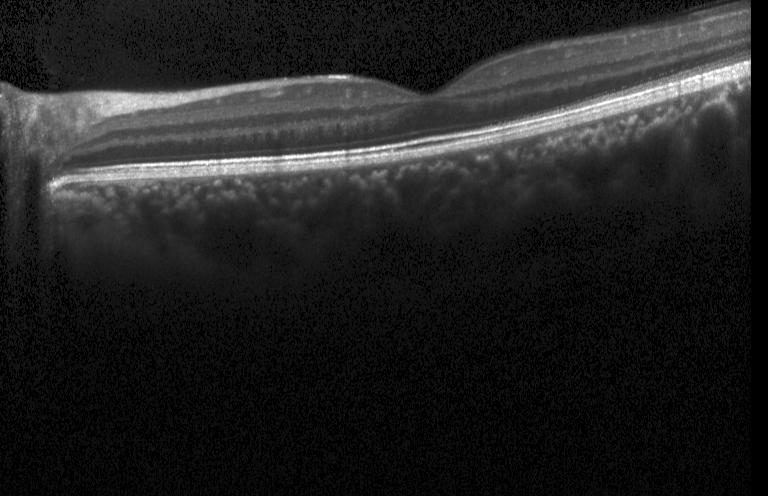 OCT B-scan · spectral-domain OCT — This B-scan demonstrates no CNV, no DME, and no drusen.